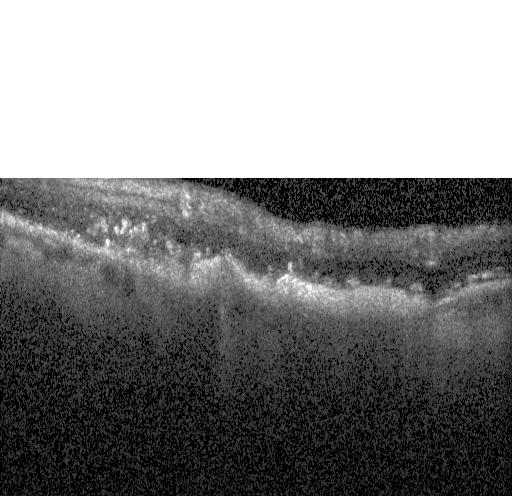 Through the macula · optical coherence tomography B-scan · acquired on a Heidelberg Spectralis · spectral-domain optical coherence tomography. The scan shows a choroidal neovascular membrane.